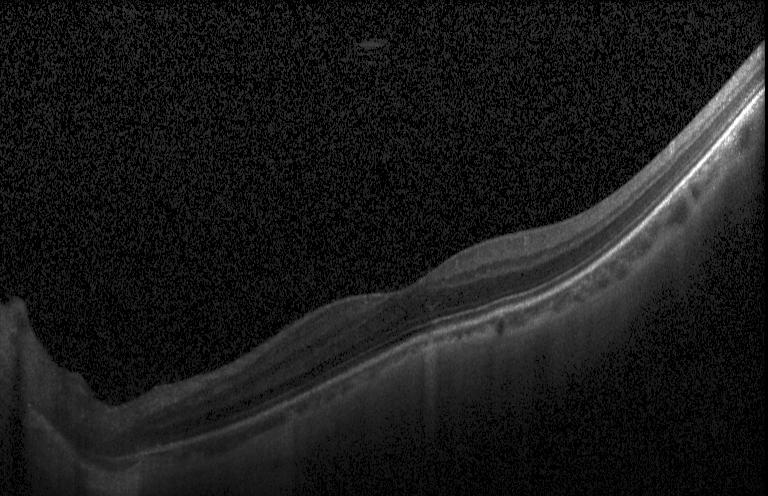 Macular OCT: neither CNV, DME, nor drusen.